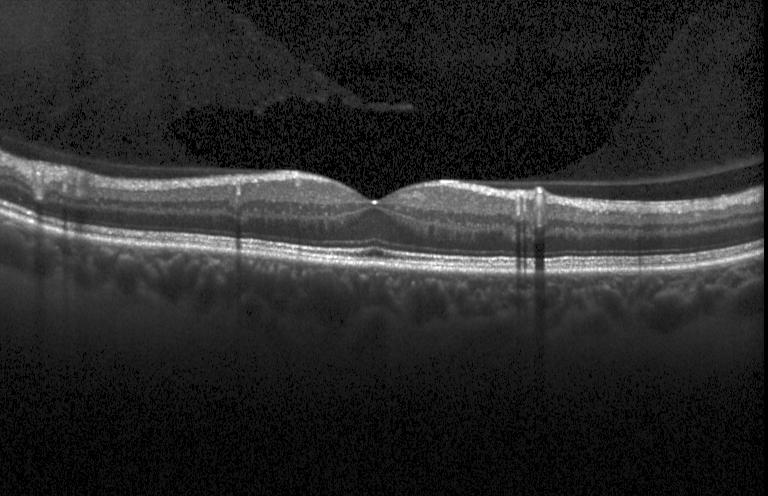
Optical coherence tomography B-scan.
This B-scan demonstrates no choroidal neovascularization, no diabetic macular edema, and no drusen.